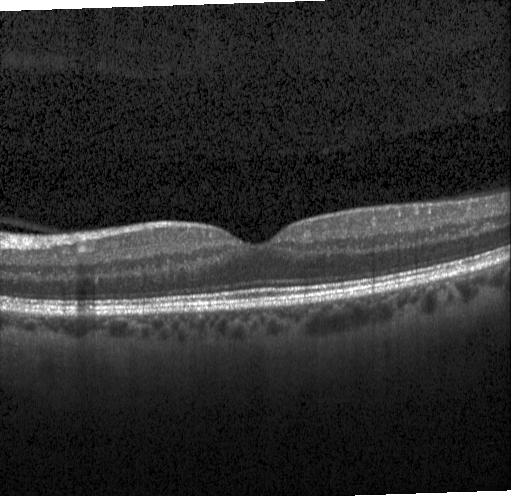 Fovea-centered · optical coherence tomography scan · SD-OCT. Diagnosis: no CNV, DME, or drusen.